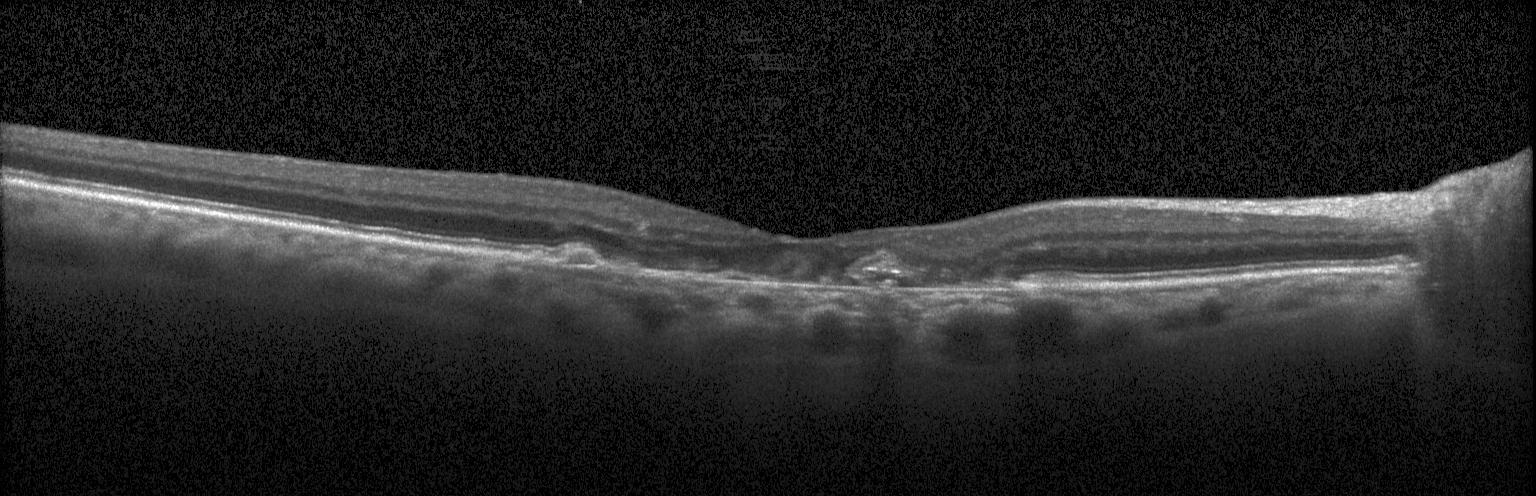
Macular OCT demonstrating a choroidal neovascular membrane.